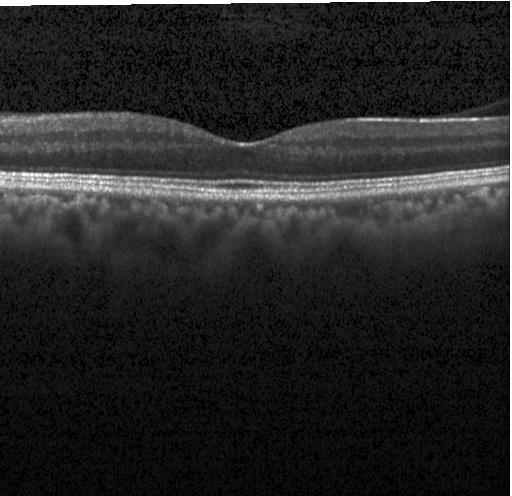

Horizontal scan through the fovea; OCT line scan; spectral-domain optical coherence tomography; acquired on a Heidelberg Spectralis
Diagnosis: no evidence of choroidal neovascularization, diabetic macular edema, or drusen.